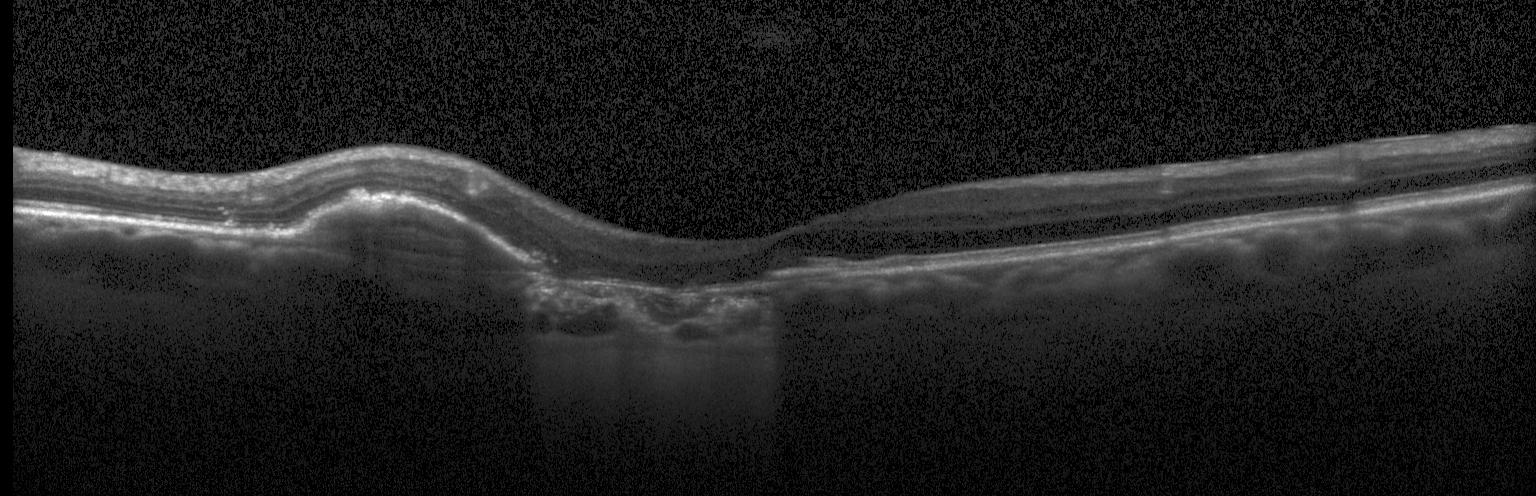
This B-scan demonstrates a choroidal neovascular membrane.